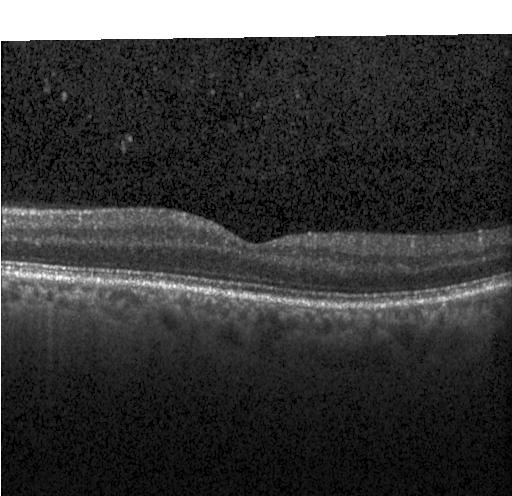 Through the macula. Acquired on a Heidelberg Spectralis. Spectral-domain OCT. Optical coherence tomography scan
Impression: no choroidal neovascularization, diabetic macular edema, or drusen.